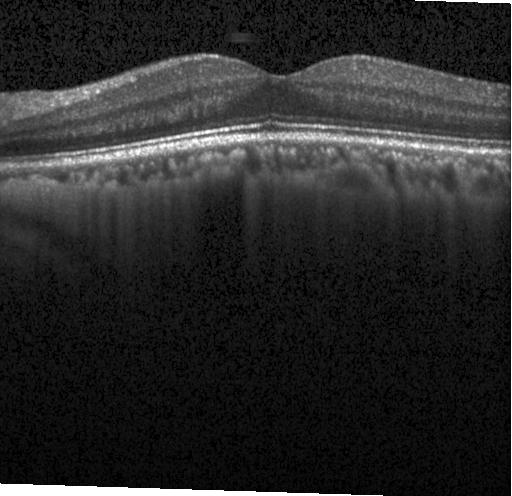
No choroidal neovascularization, diabetic macular edema, or drusen.